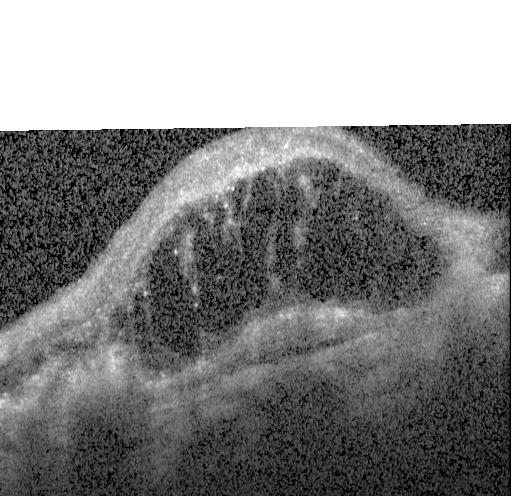
Spectral-domain optical coherence tomography; OCT line scan; Heidelberg Spectralis OCT system; macular scan. Finding: diabetic macular edema (DME).